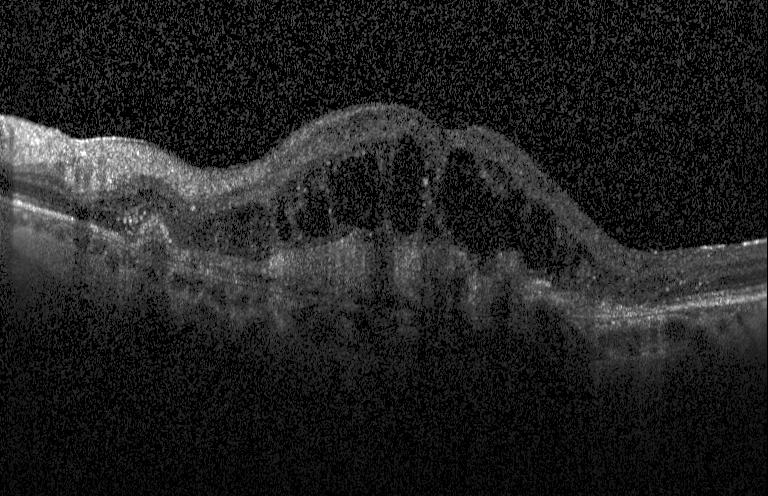 Spectral-domain OCT; optical coherence tomography scan. A choroidal neovascular membrane.